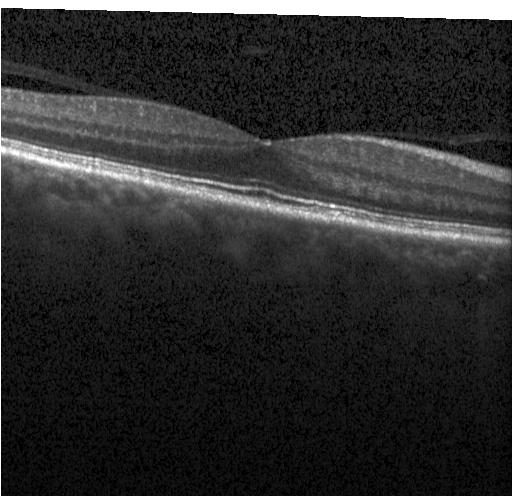

Retinal OCT B-scan · Heidelberg Spectralis OCT system · through the macula
Impression: neither choroidal neovascularization, diabetic macular edema, nor drusen.